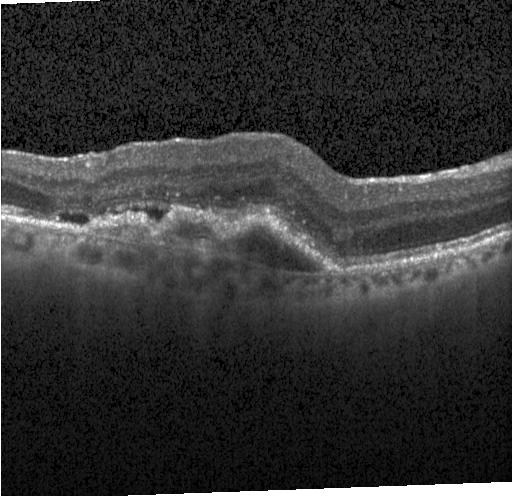

Retinal OCT cross-section showing a choroidal neovascular membrane.